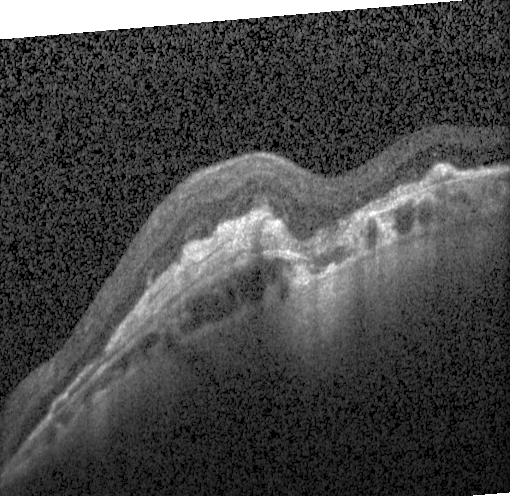

Finding: a choroidal neovascular membrane.